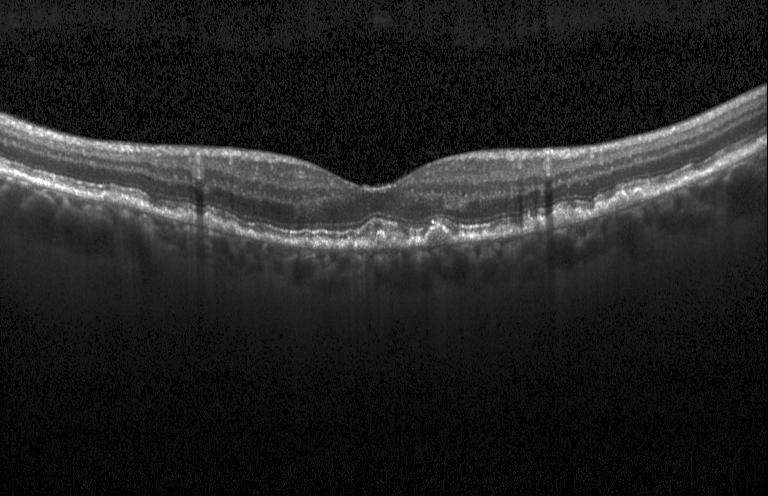
OCT B-scan.
Multiple drusen.